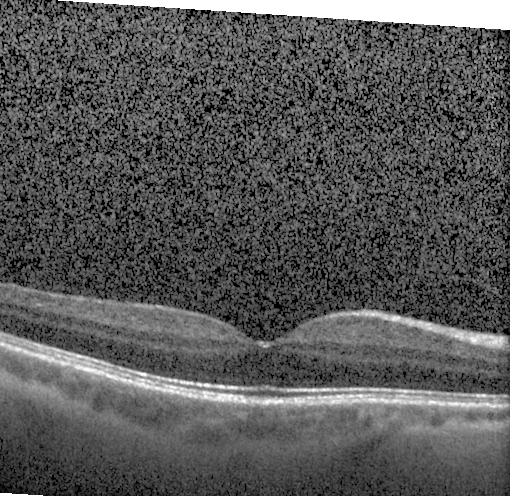 Acquired on a Heidelberg Spectralis, macular scan, retinal OCT B-scan, SD-OCT — This B-scan demonstrates no evidence of choroidal neovascularization, diabetic macular edema, or drusen.